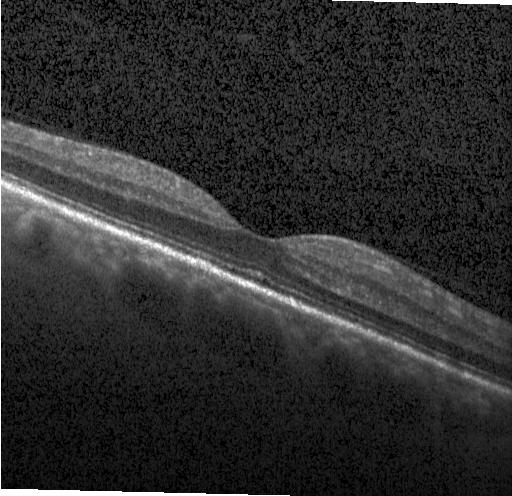

This B-scan demonstrates neither CNV, DME, nor drusen.